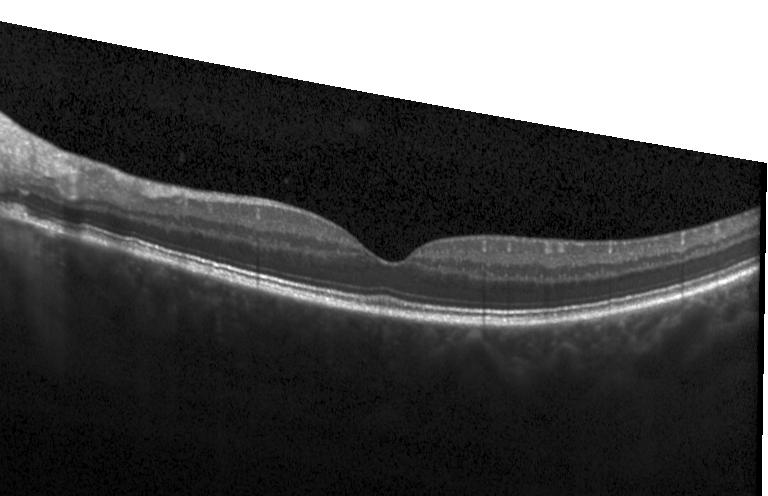 OCT B-scan. Instrument: Heidelberg Spectralis.
This B-scan demonstrates no choroidal neovascularization, diabetic macular edema, or drusen.